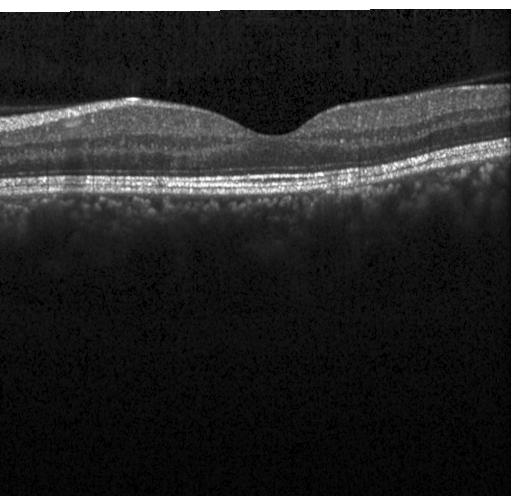

OCT B-scan — Macular OCT: no evidence of choroidal neovascularization, diabetic macular edema, or drusen.